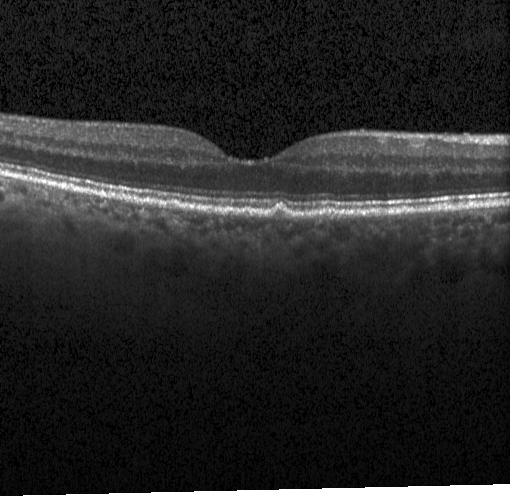
Diagnosis: sub-RPE drusenoid deposits.